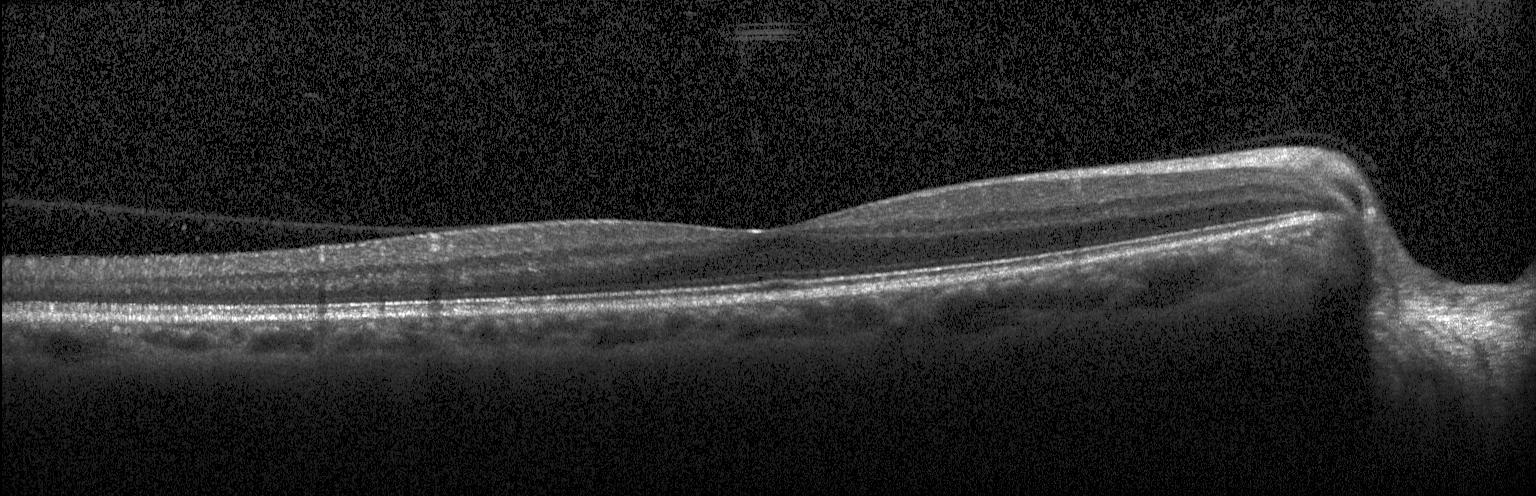
Dx: no evidence of choroidal neovascularization, diabetic macular edema, or drusen.